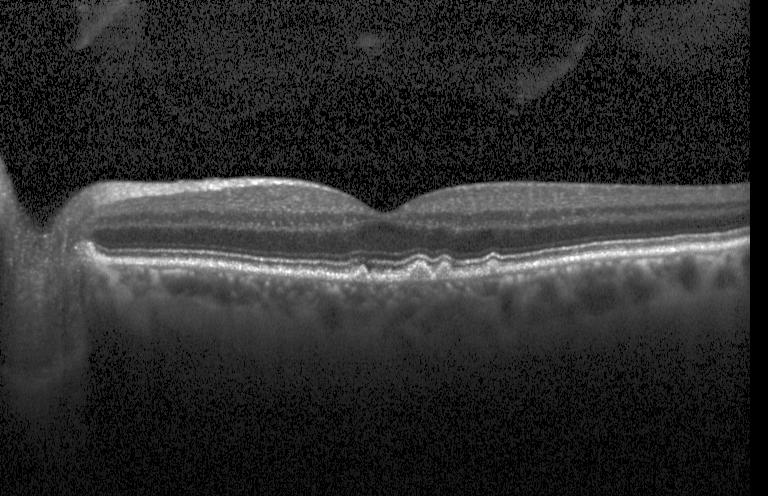
Instrument: Heidelberg Spectralis, retinal OCT B-scan, SD-OCT.
This B-scan demonstrates drusen.